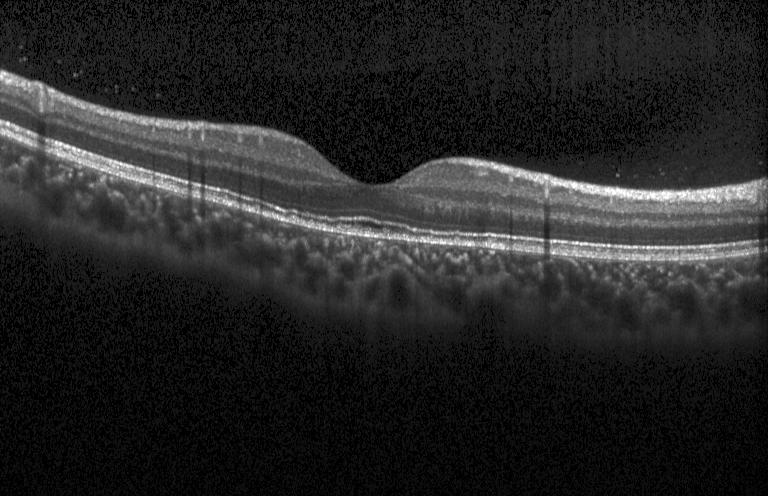 Macular scan · SD-OCT · instrument: Heidelberg Spectralis · OCT line scan
Impression: neither choroidal neovascularization, diabetic macular edema, nor drusen.